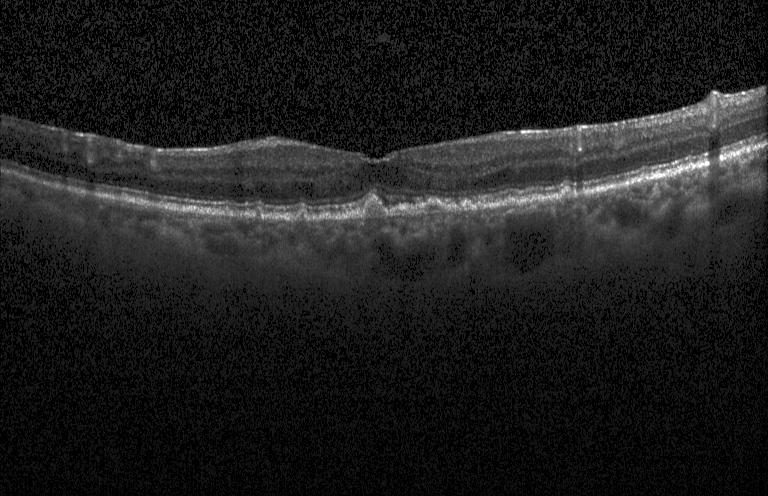 Centered on the fovea. OCT line scan. Heidelberg Spectralis.
Finding: multiple drusen.